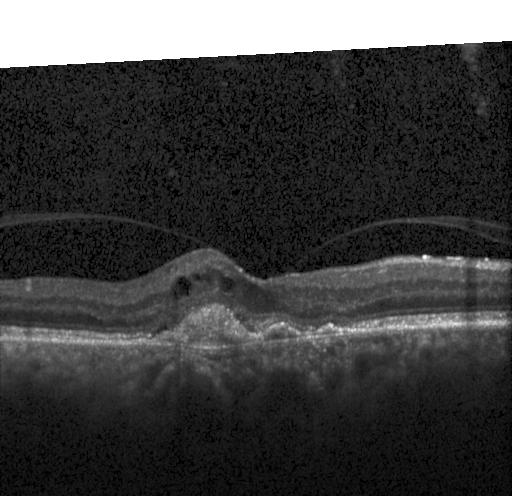 Through the macula · optical coherence tomography scan · Heidelberg Spectralis · spectral-domain OCT. The scan shows a choroidal neovascular membrane.